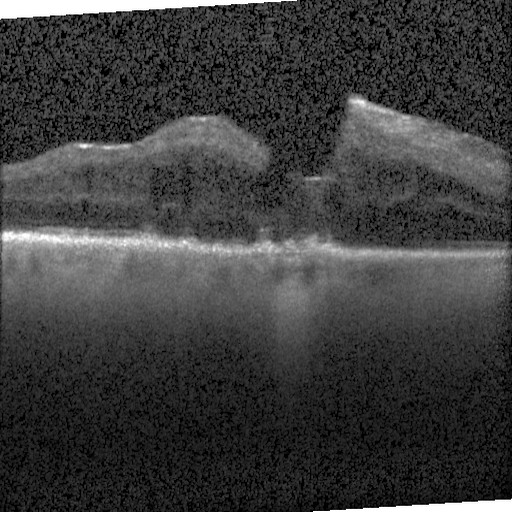

Impression: diabetic macular edema (DME).